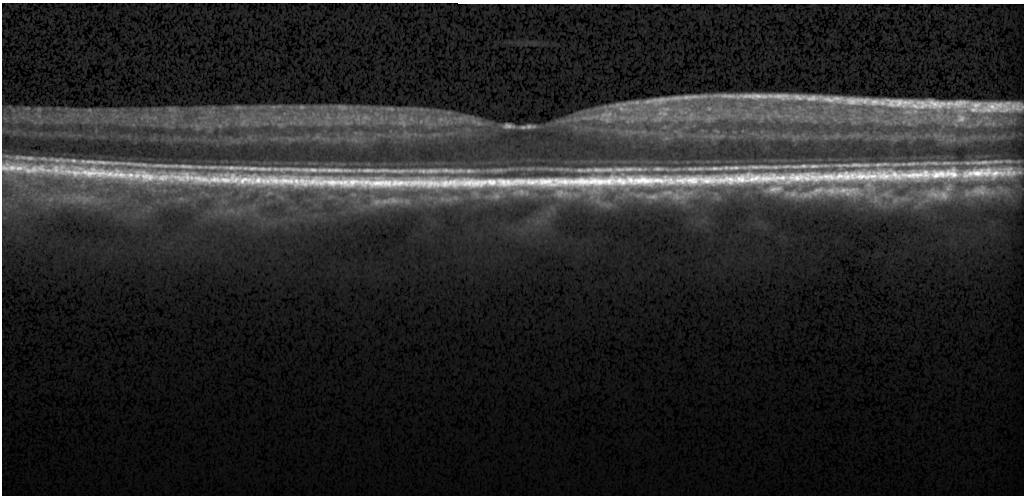
Diagnosis: no choroidal neovascularization, diabetic macular edema, or drusen.